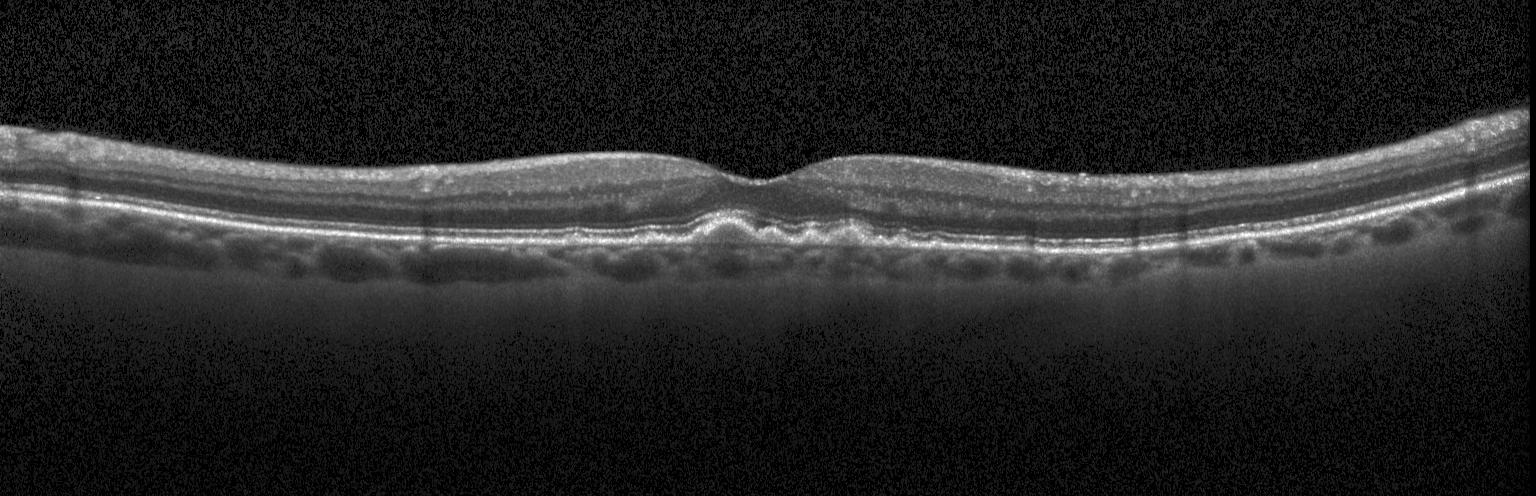
Drusen.